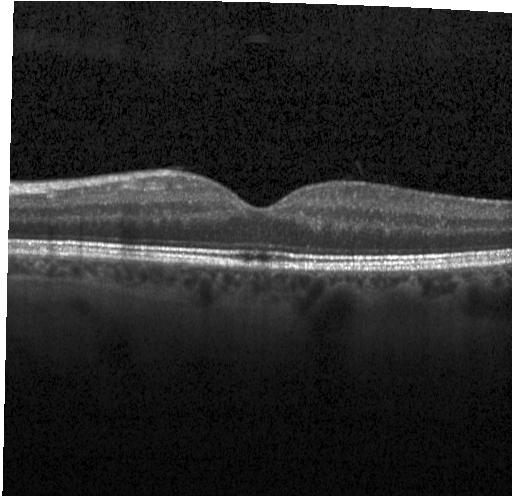

Retinal OCT B-scan — Macular OCT: no CNV, DME, or drusen.